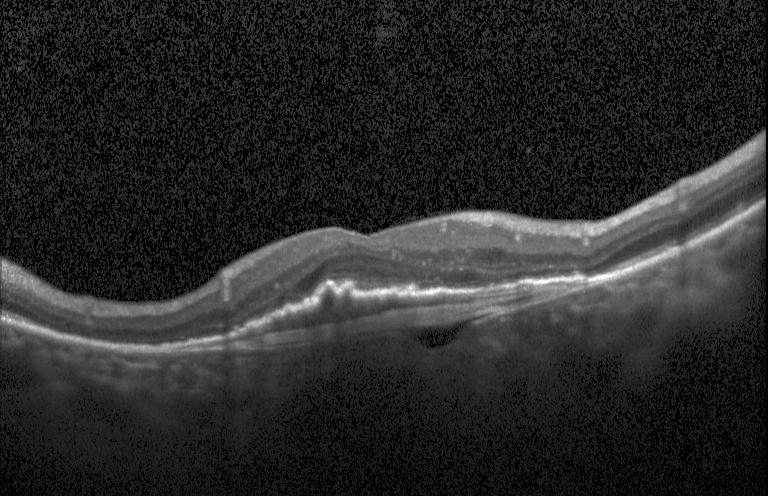

Macular OCT demonstrating a choroidal neovascular membrane.